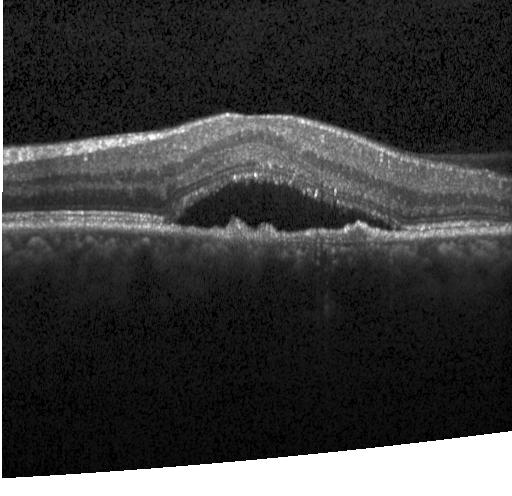 Heidelberg Spectralis OCT system · SD-OCT · OCT B-scan. Finding: a choroidal neovascular membrane.